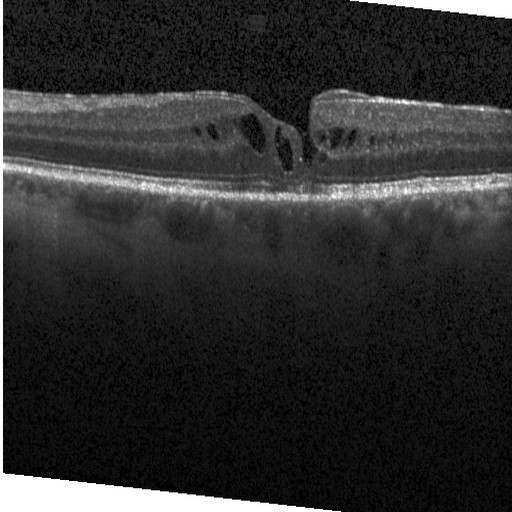
Horizontal scan through the fovea · SD-OCT · retinal OCT B-scan
Impression: DME.